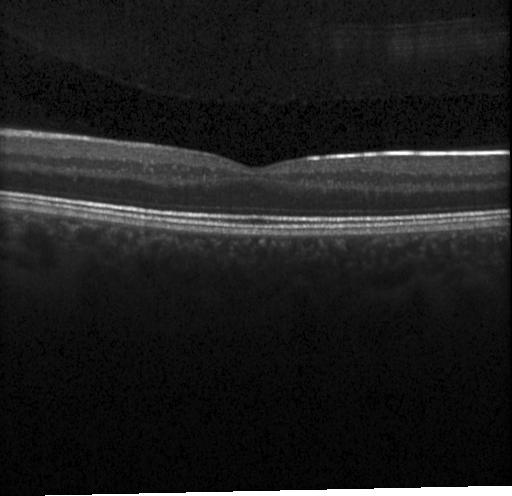 Retinal OCT B-scan; spectral-domain OCT. Impression: neither CNV, DME, nor drusen.